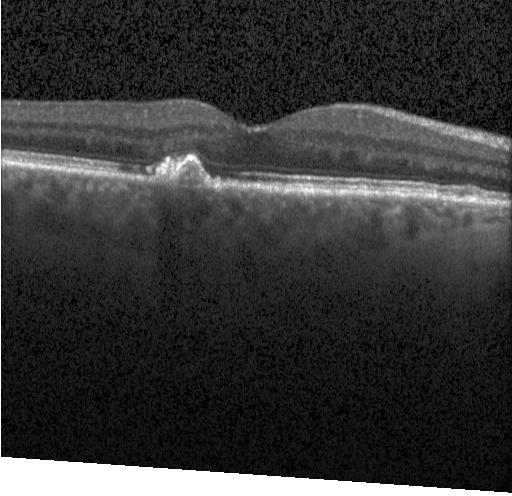
OCT line scan · spectral-domain optical coherence tomography · acquired on a Heidelberg Spectralis. Impression: CNV.